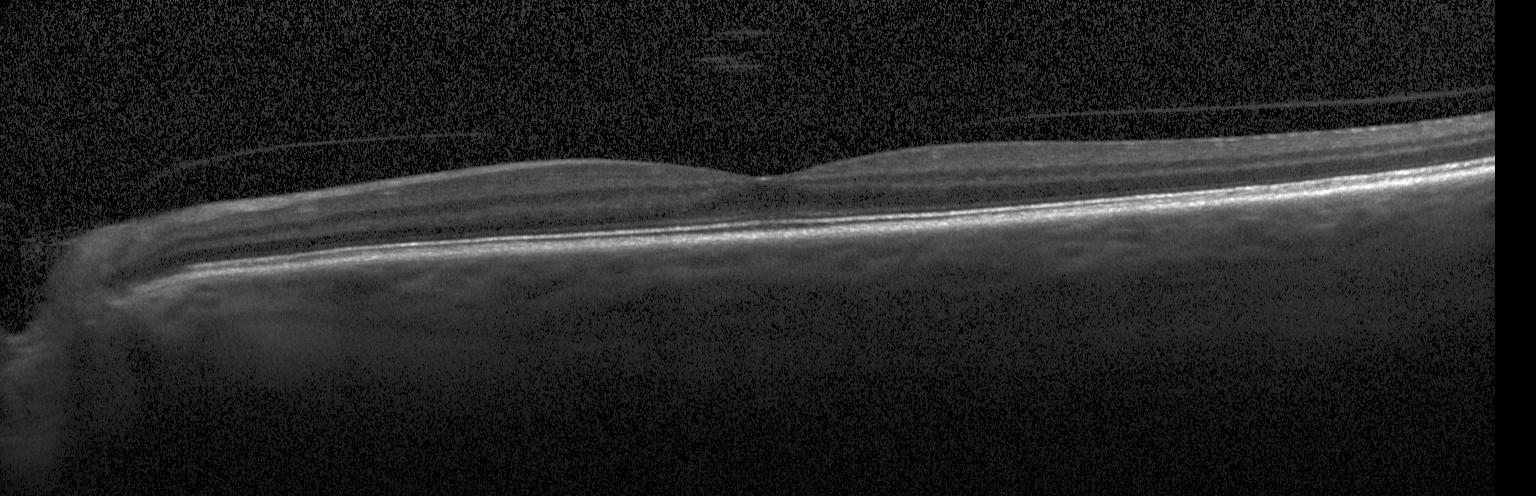
Retinal OCT cross-section. No evidence of CNV, DME, or drusen.